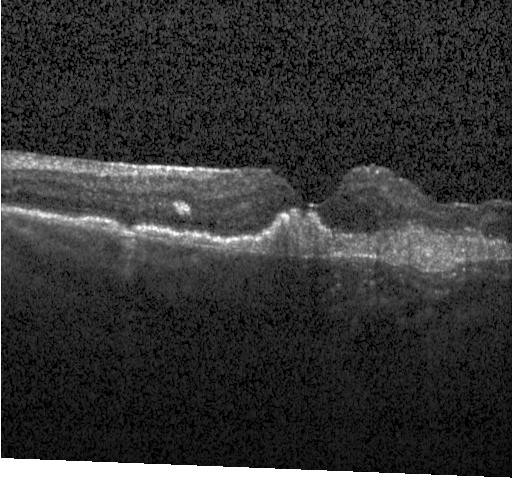
Retinal OCT cross-section. Heidelberg Spectralis. SD-OCT.
OCT finding: a choroidal neovascular membrane.